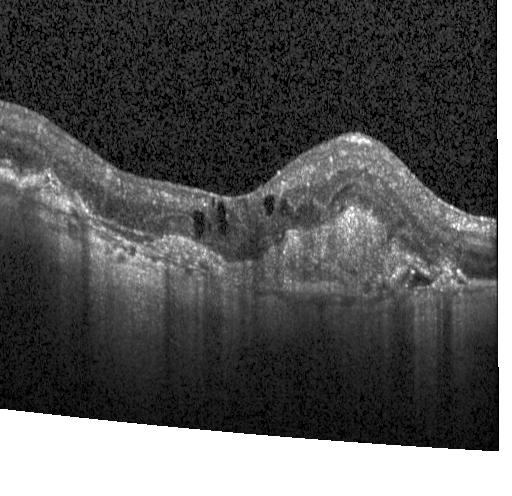

OCT B-scan showing choroidal neovascularization.